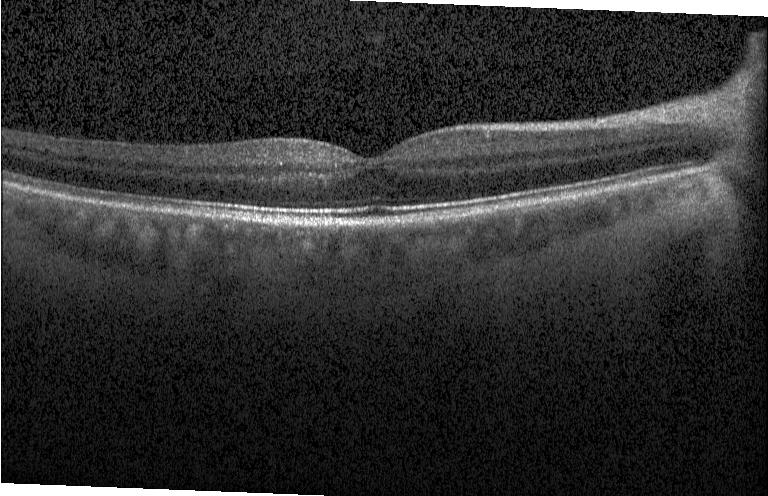

Retinal OCT B-scan. Horizontal scan through the fovea. OCT finding: no evidence of choroidal neovascularization, diabetic macular edema, or drusen.